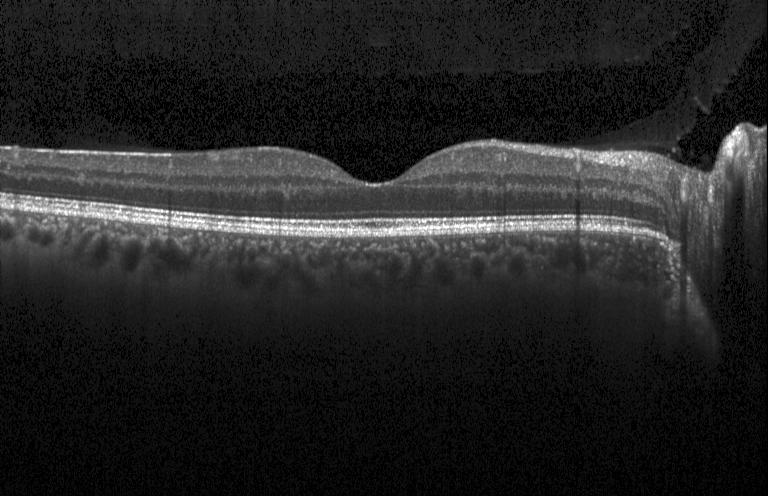

Retinal OCT B-scan; macular scan; spectral-domain optical coherence tomography — Finding: no choroidal neovascularization, diabetic macular edema, or drusen.